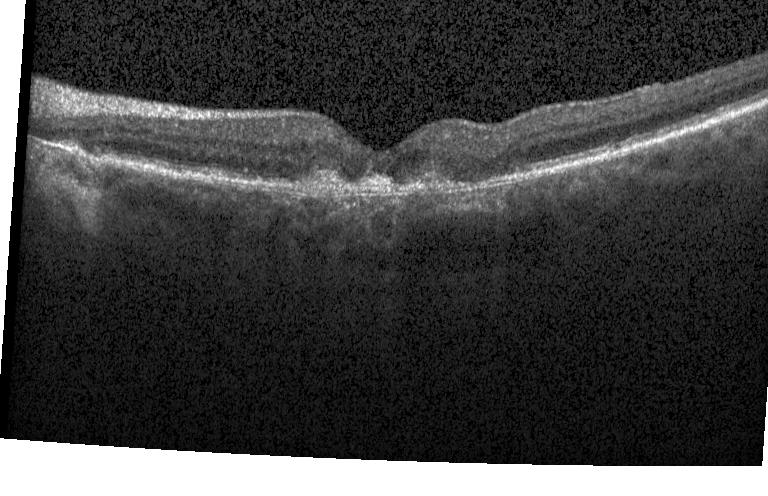 OCT scan showing choroidal neovascularization (CNV).